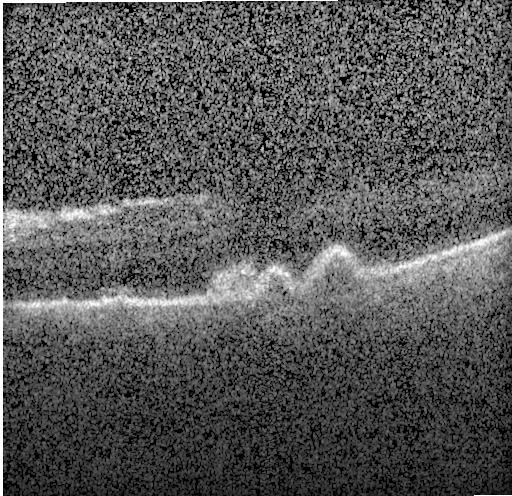 OCT line scan. Heidelberg Spectralis OCT system. Centered on the fovea. Finding: sub-RPE drusenoid deposits.